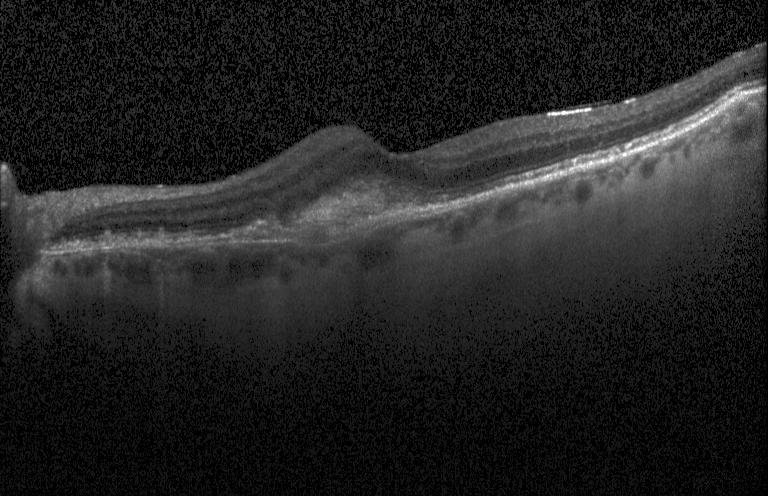
Retinal OCT B-scan, through the macula
Macular OCT: a choroidal neovascular membrane.